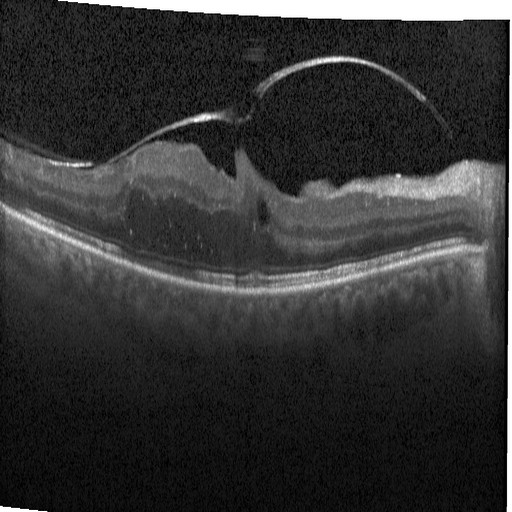 Optical coherence tomography scan. The scan shows diabetic macular edema.